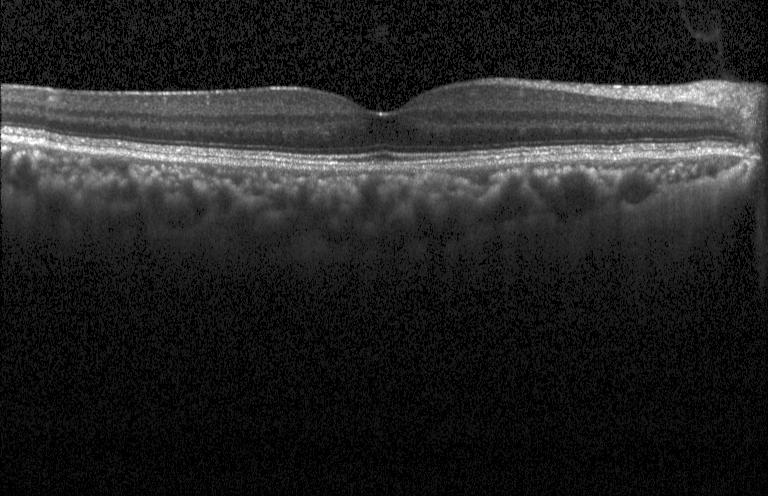 OCT finding: neither choroidal neovascularization, diabetic macular edema, nor drusen.